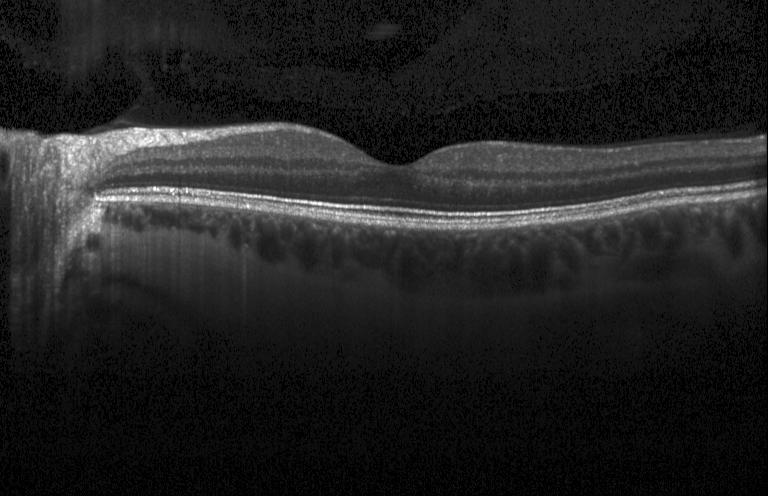
OCT line scan; centered on the fovea; instrument: Heidelberg Spectralis.
Assessment: no evidence of choroidal neovascularization, diabetic macular edema, or drusen.